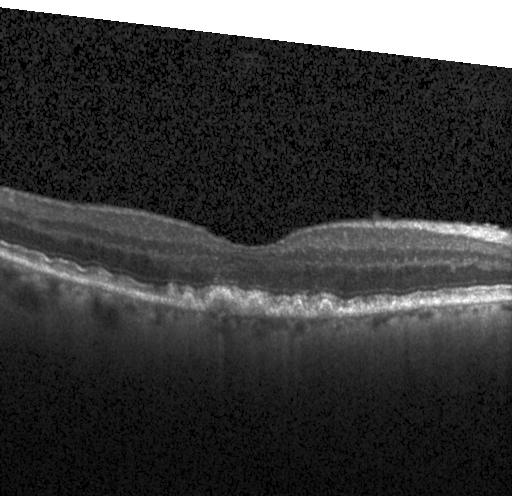
Macular scan · retinal OCT cross-section · spectral-domain OCT · Heidelberg Spectralis OCT system — Impression: drusen.